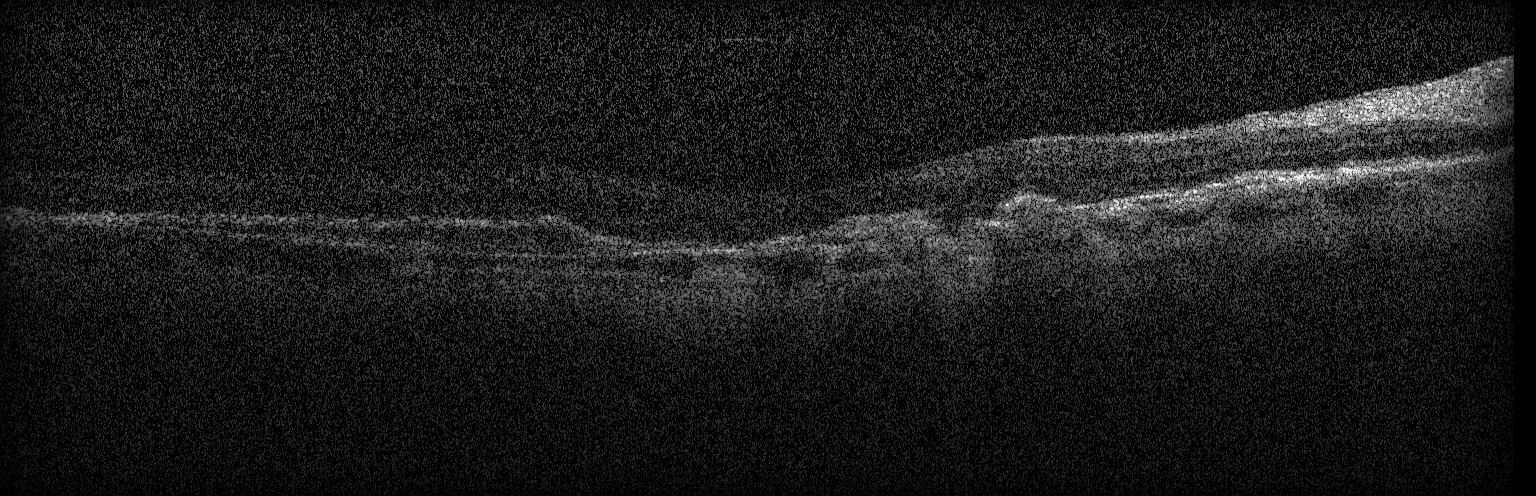 Diagnosis: a choroidal neovascular membrane.